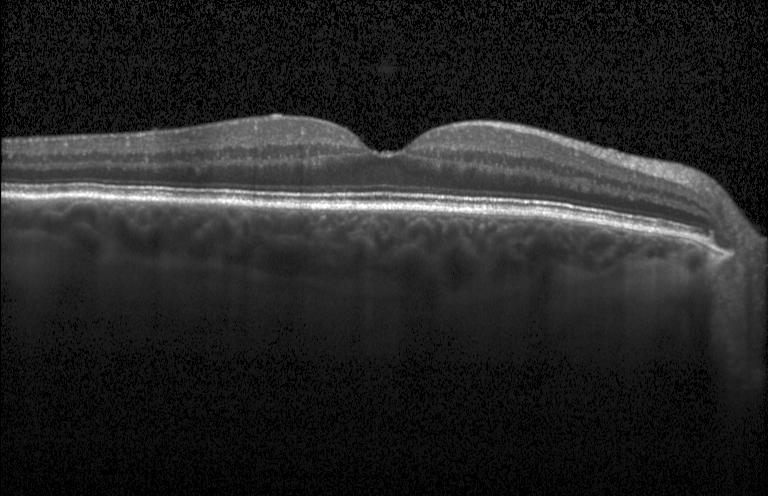 Finding: neither CNV, DME, nor drusen.